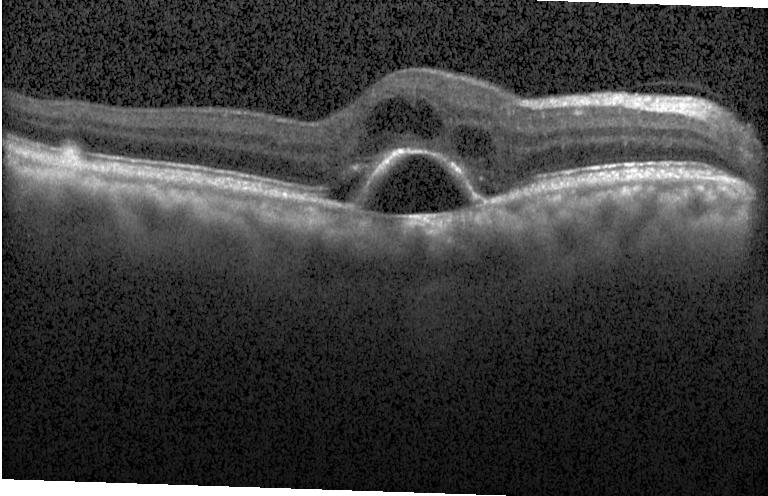 Optical coherence tomography B-scan. A choroidal neovascular membrane.